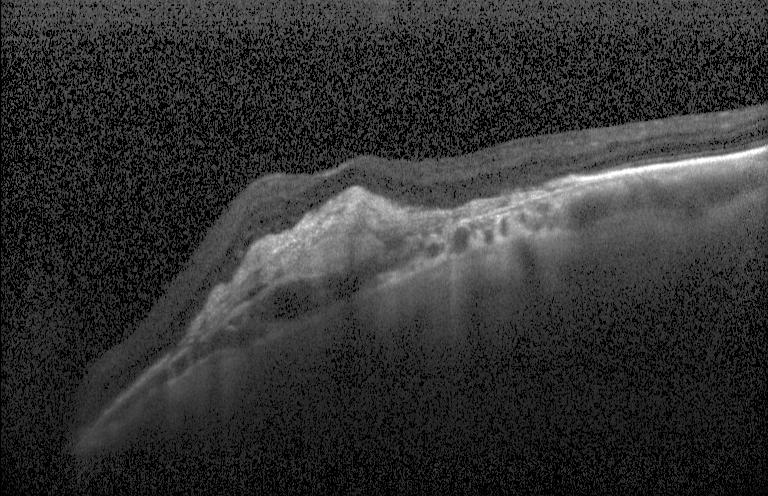

Choroidal neovascularization (CNV).